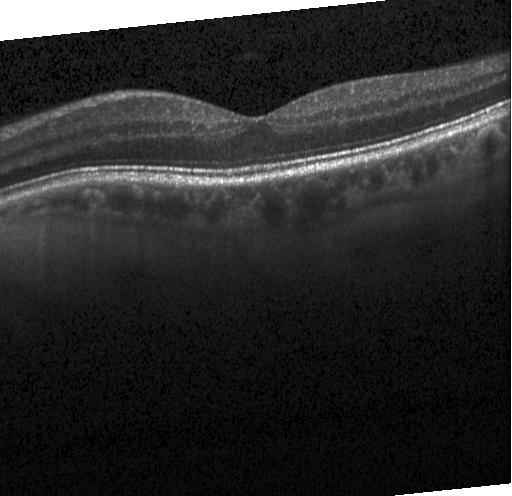
Impression: no evidence of CNV, DME, or drusen.